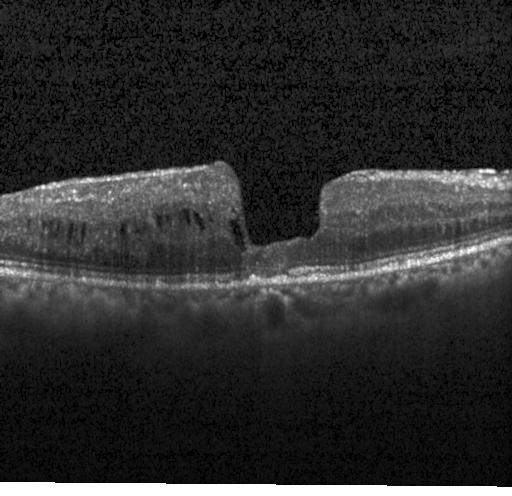

Assessment: diabetic macular edema.